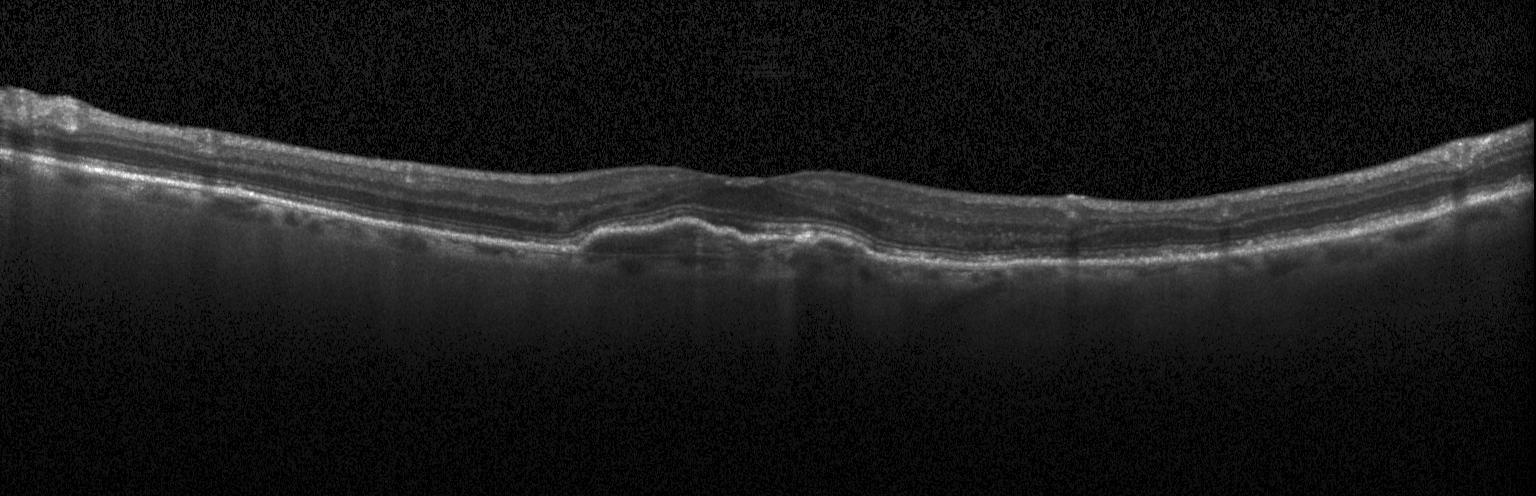
Optical coherence tomography scan.
Diagnosis: a choroidal neovascular membrane.